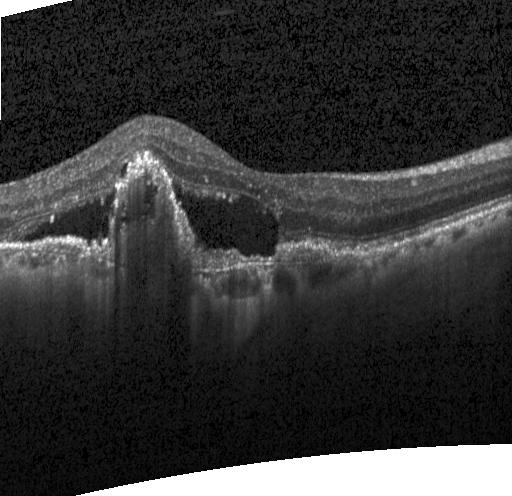 Macular scan. OCT B-scan
This B-scan demonstrates CNV.